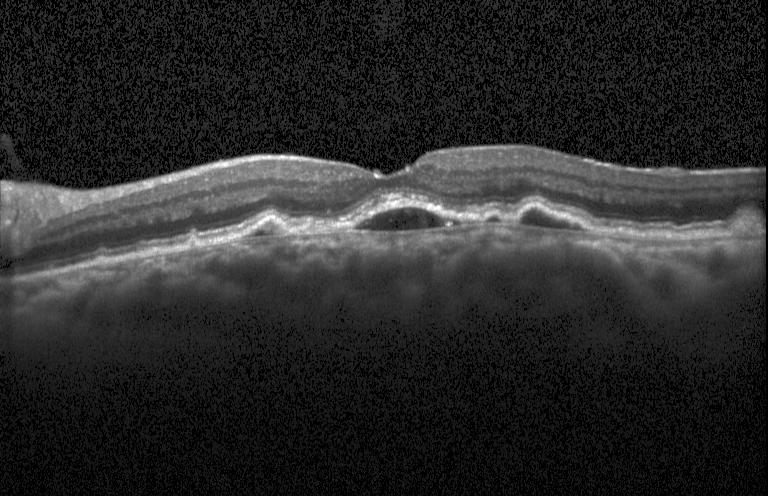
Heidelberg Spectralis · optical coherence tomography scan.
The scan shows a choroidal neovascular membrane.